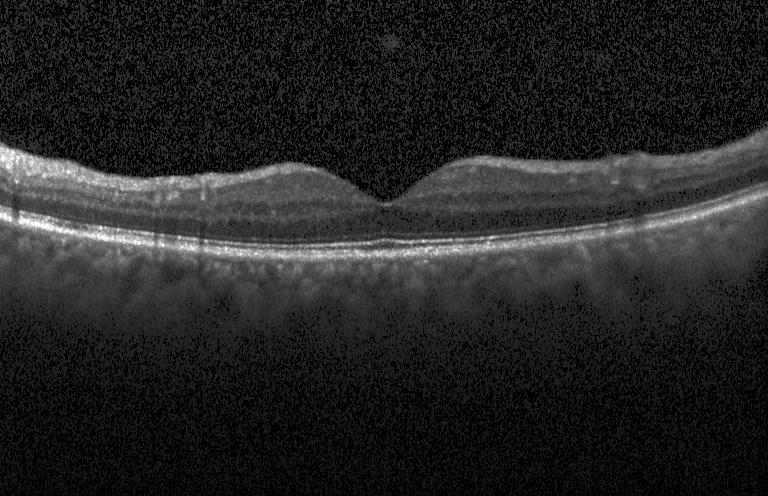
Macular OCT: neither choroidal neovascularization, diabetic macular edema, nor drusen.